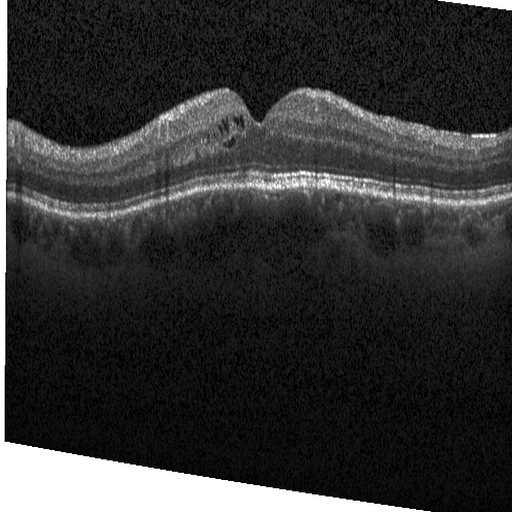 Diagnosis: diabetic macular edema.